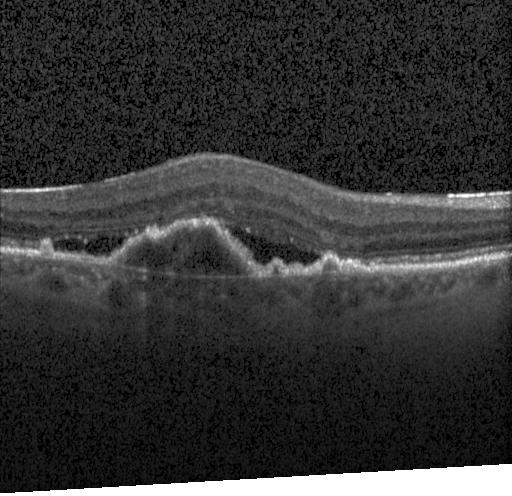

OCT scan showing a choroidal neovascular membrane.